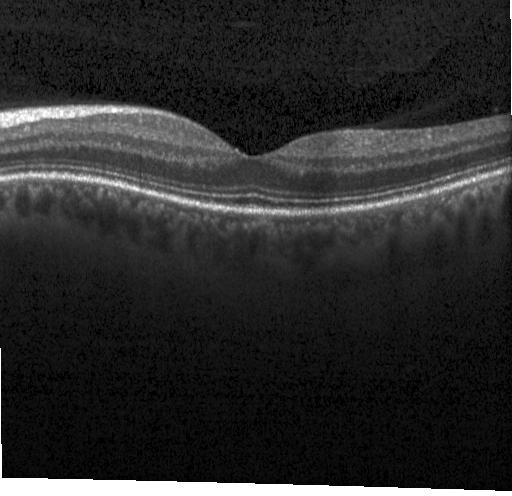
Spectral-domain OCT, macular scan, optical coherence tomography scan
Macular OCT: no choroidal neovascularization, no diabetic macular edema, and no drusen.